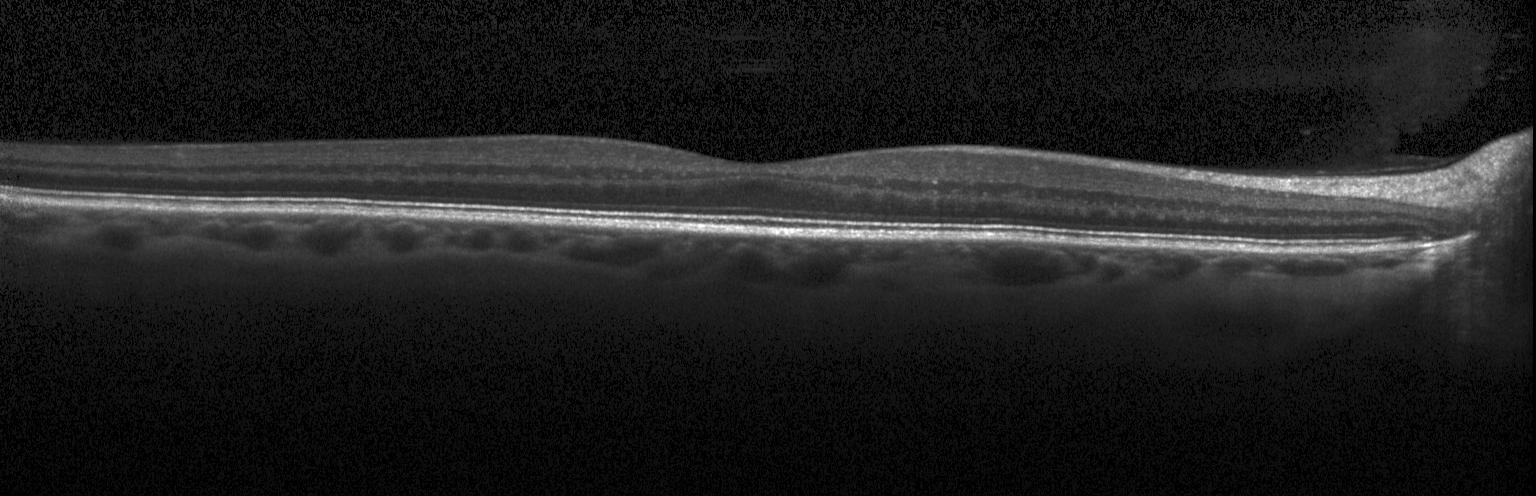
Through the macula · Heidelberg Spectralis OCT system · spectral-domain optical coherence tomography · optical coherence tomography B-scan
The scan shows neither CNV, DME, nor drusen.